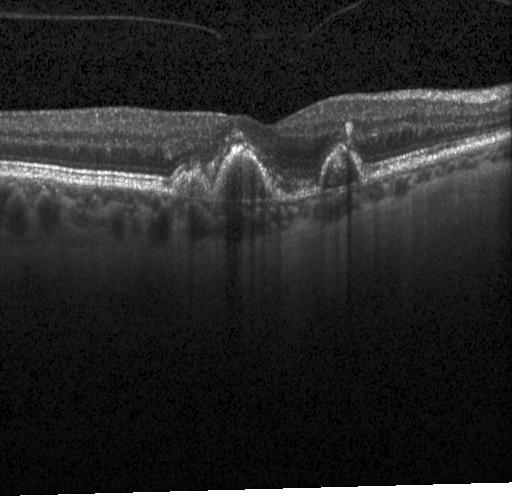 Choroidal neovascularization (CNV).